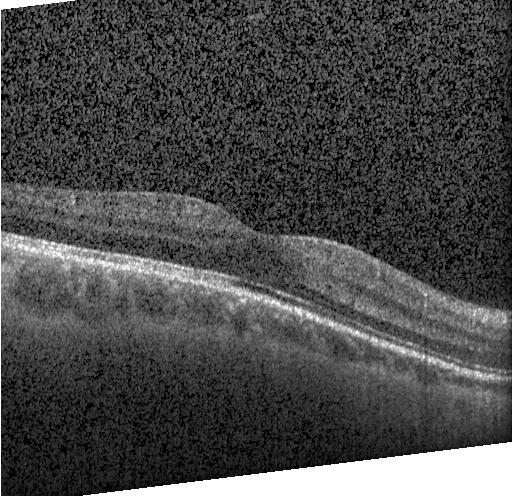

OCT B-scan — Finding: no choroidal neovascularization, no diabetic macular edema, and no drusen.